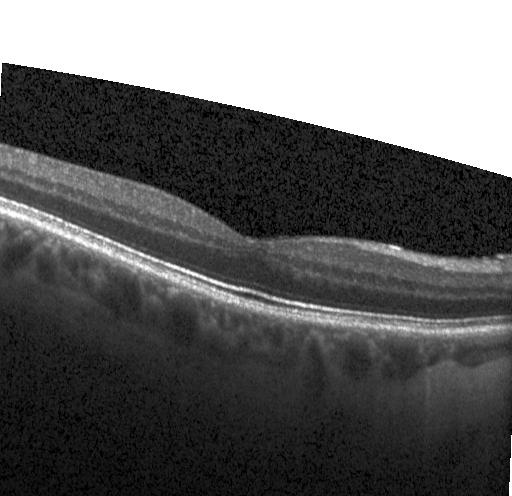

OCT line scan.
Assessment: no choroidal neovascularization, no diabetic macular edema, and no drusen.